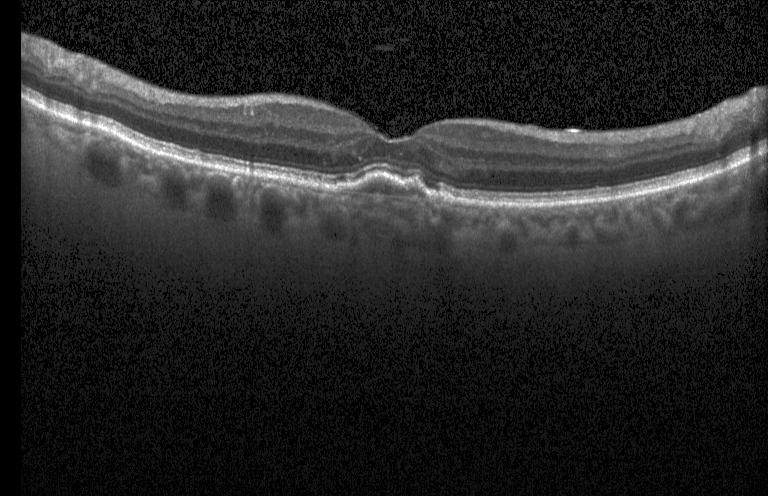 OCT B-scan showing choroidal neovascularization (CNV).